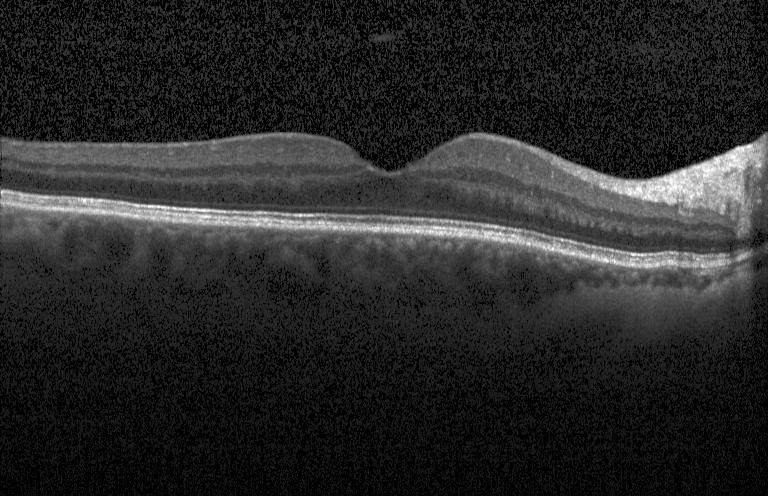
OCT finding: no CNV, no DME, and no drusen.